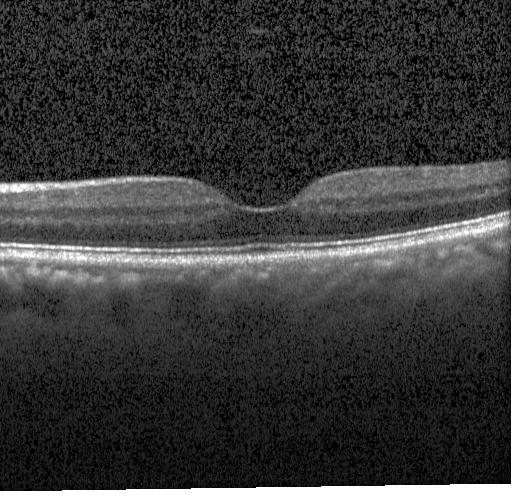

Retinal OCT B-scan. Impression: no CNV, DME, or drusen.